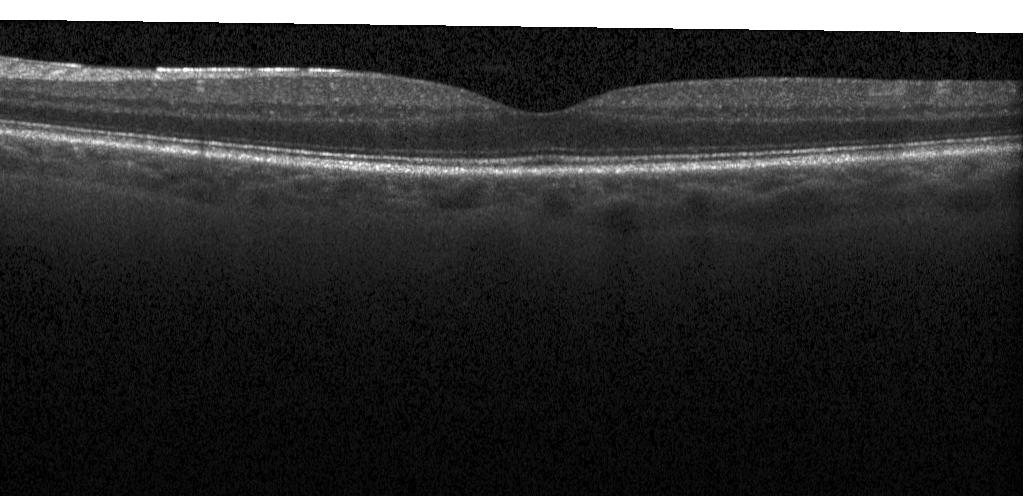

OCT line scan. Fovea-centered. Diagnosis: neither CNV, DME, nor drusen.